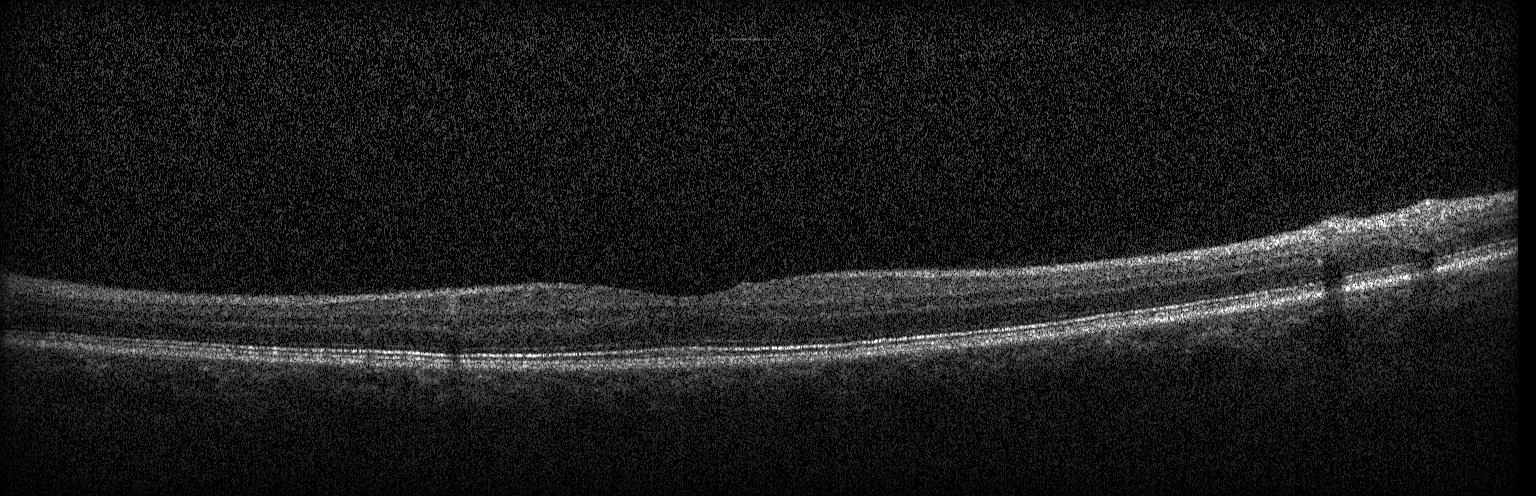 Assessment: neither choroidal neovascularization, diabetic macular edema, nor drusen.